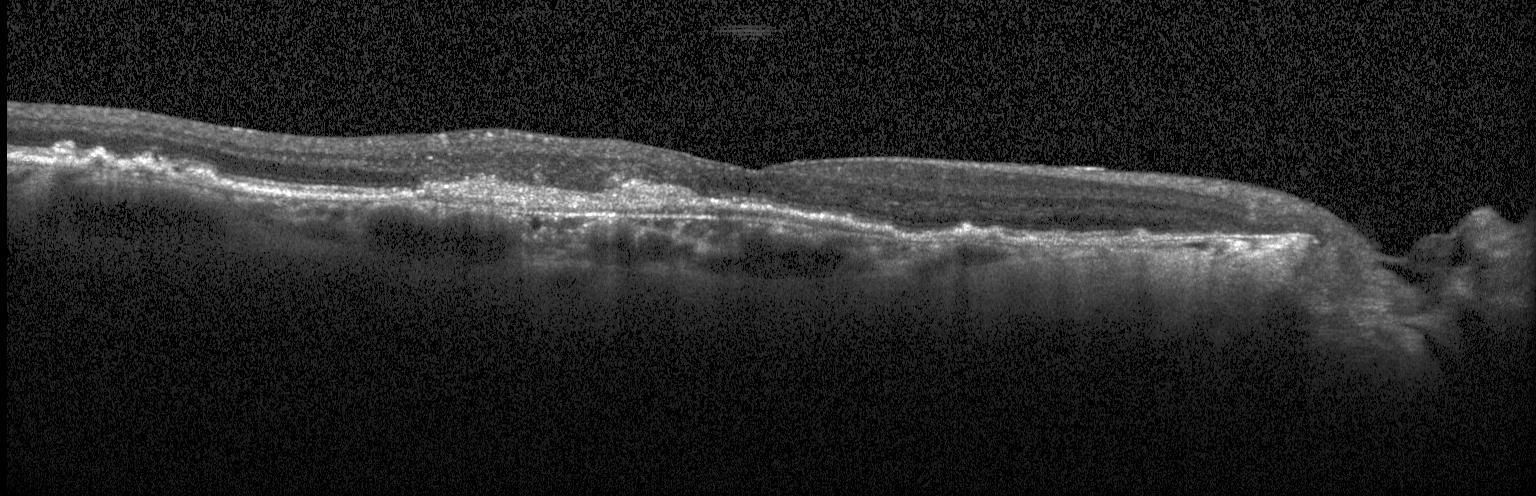
Optical coherence tomography scan
Impression: choroidal neovascularization.